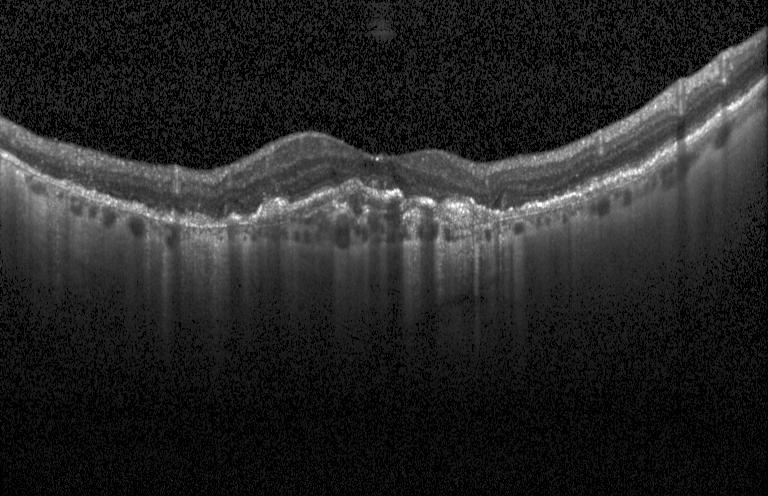

Macular scan; spectral-domain optical coherence tomography; OCT line scan.
Impression: a choroidal neovascular membrane.